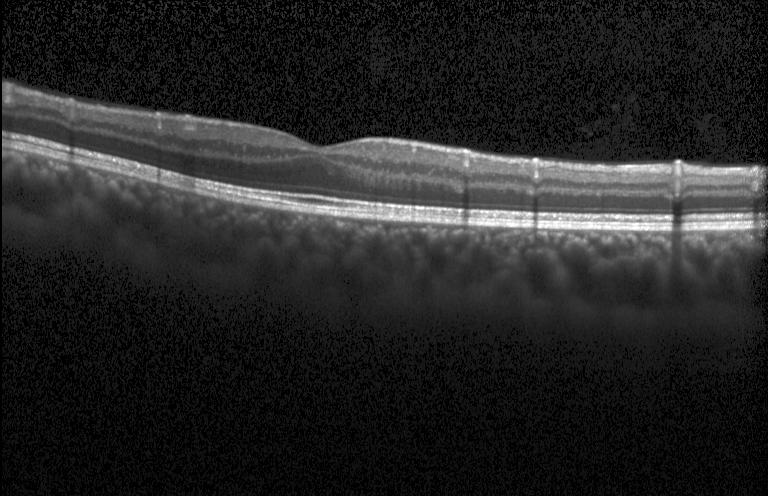
Macular OCT demonstrating neither CNV, DME, nor drusen.